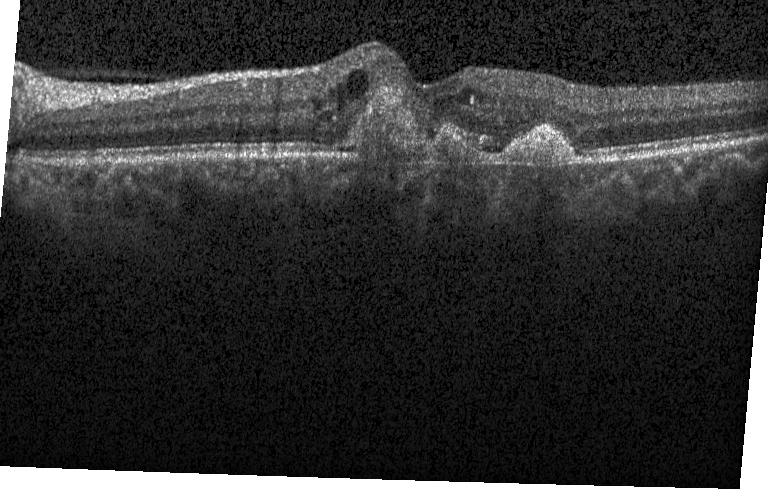
Dx: choroidal neovascularization (CNV).